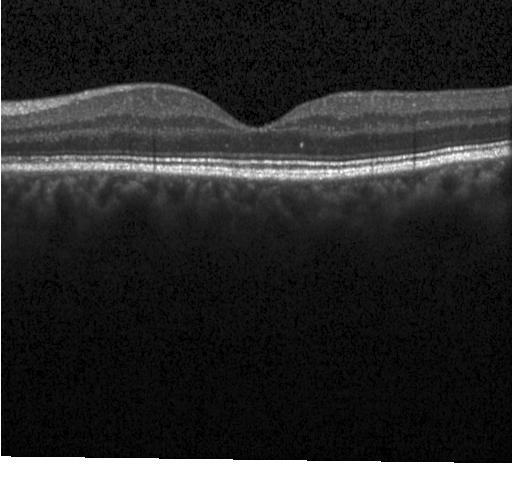 Retinal OCT cross-section
Assessment: no choroidal neovascularization, diabetic macular edema, or drusen.